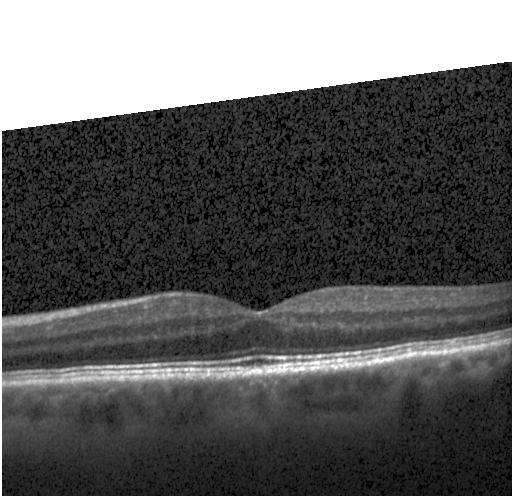

OCT B-scan. Spectral-domain OCT. Horizontal scan through the fovea. Instrument: Heidelberg Spectralis. Macular OCT: neither CNV, DME, nor drusen.